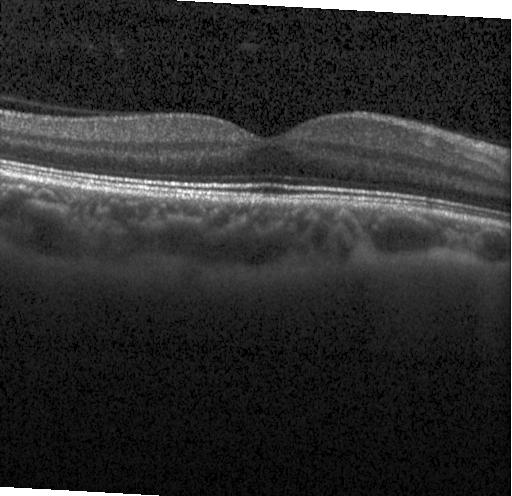

Macular OCT: no choroidal neovascularization, diabetic macular edema, or drusen.